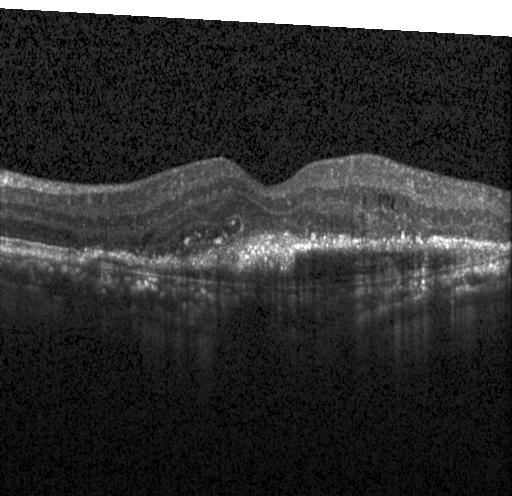

Retinal OCT cross-section; acquired on a Heidelberg Spectralis; SD-OCT.
OCT finding: a choroidal neovascular membrane.